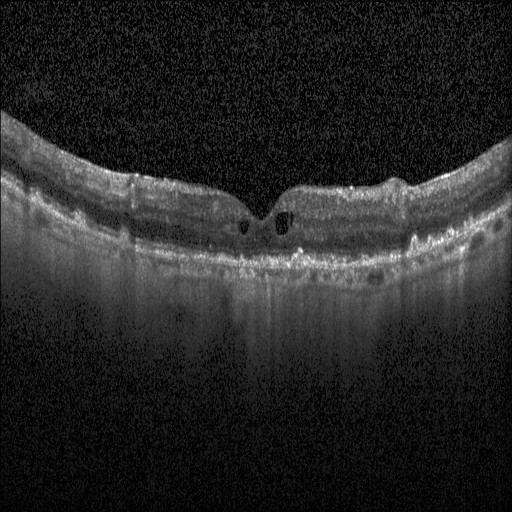 Heidelberg Spectralis; OCT B-scan.
Assessment: diabetic macular edema.